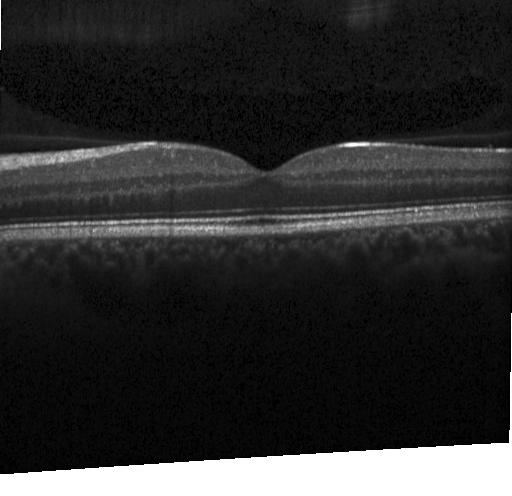
Horizontal scan through the fovea · retinal OCT B-scan · spectral-domain optical coherence tomography — Macular OCT: no CNV, DME, or drusen.